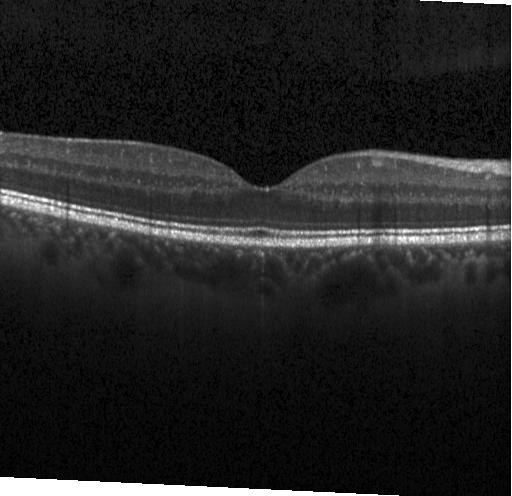

Finding: no evidence of choroidal neovascularization, diabetic macular edema, or drusen.